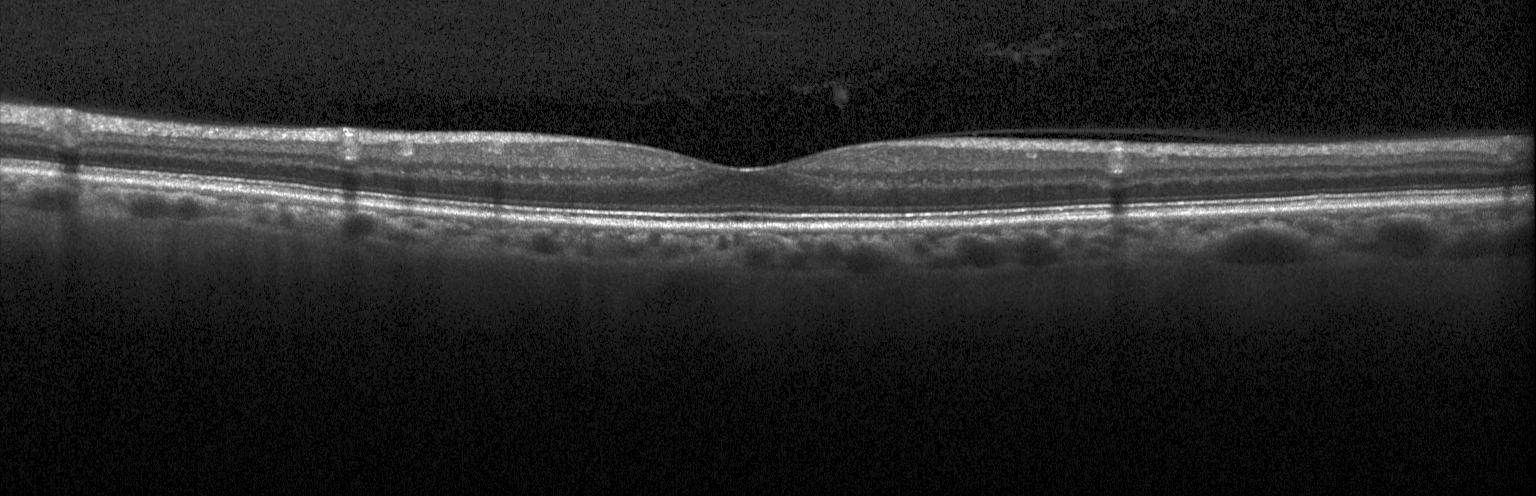
Through the macula · retinal OCT B-scan · SD-OCT · Heidelberg Spectralis
Impression: no CNV, DME, or drusen.